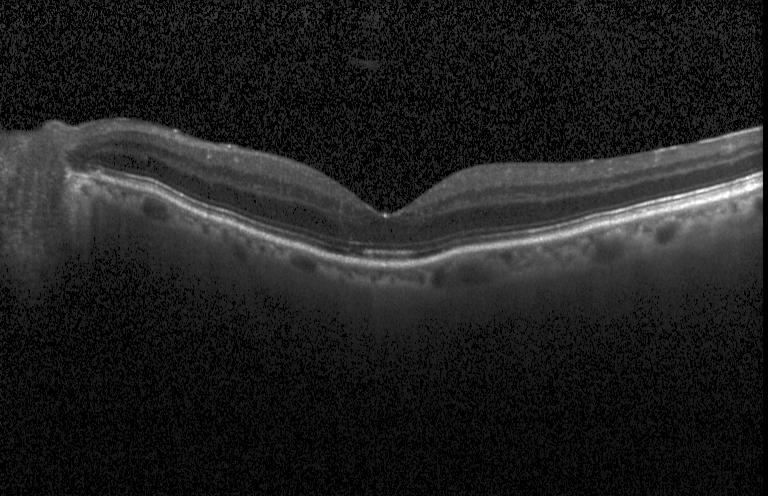 Through the macula · OCT line scan.
The scan shows neither choroidal neovascularization, diabetic macular edema, nor drusen.